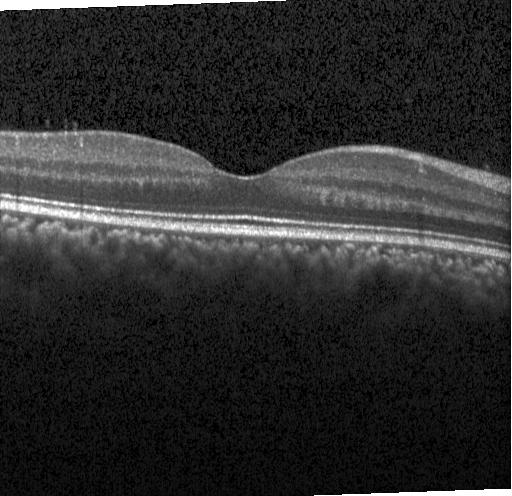

OCT finding: no CNV, no DME, and no drusen.